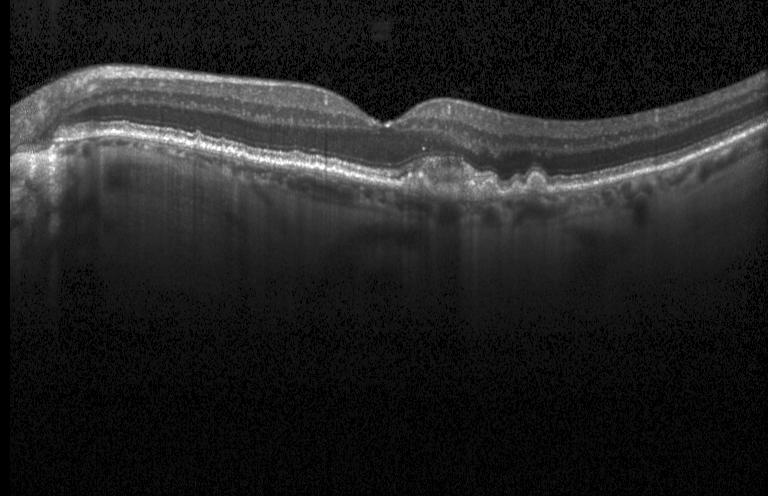 Optical coherence tomography B-scan. Assessment: CNV.